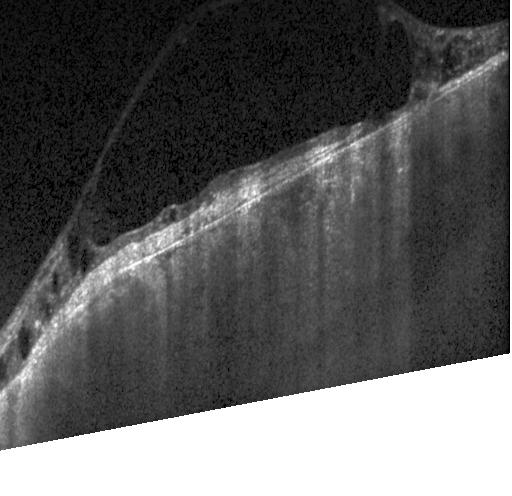 OCT B-scan. Heidelberg Spectralis OCT system. Horizontal scan through the fovea. The scan shows CNV.